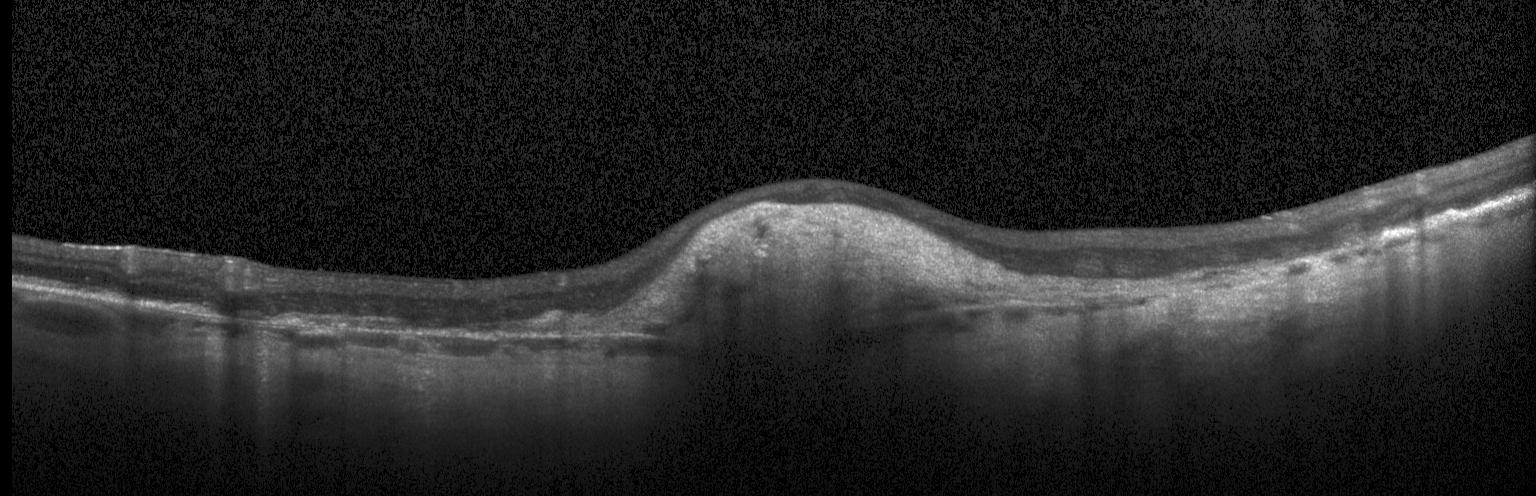

Through the macula. SD-OCT. Heidelberg Spectralis OCT system. OCT B-scan.
Dx: CNV.